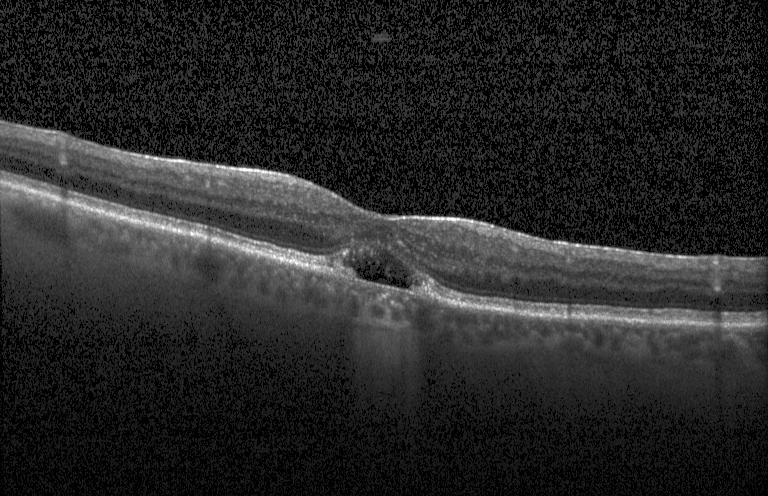
Spectral-domain OCT B-scan: a choroidal neovascular membrane.